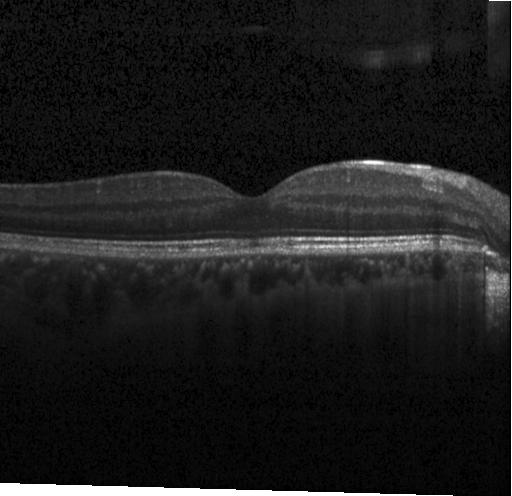

OCT line scan. Macular scan — Finding: no choroidal neovascularization, diabetic macular edema, or drusen.